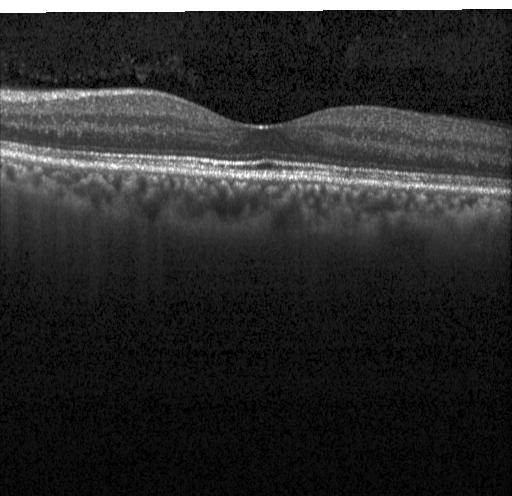
Heidelberg Spectralis OCT system, spectral-domain OCT, centered on the fovea, retinal OCT B-scan.
Assessment: no choroidal neovascularization, no diabetic macular edema, and no drusen.